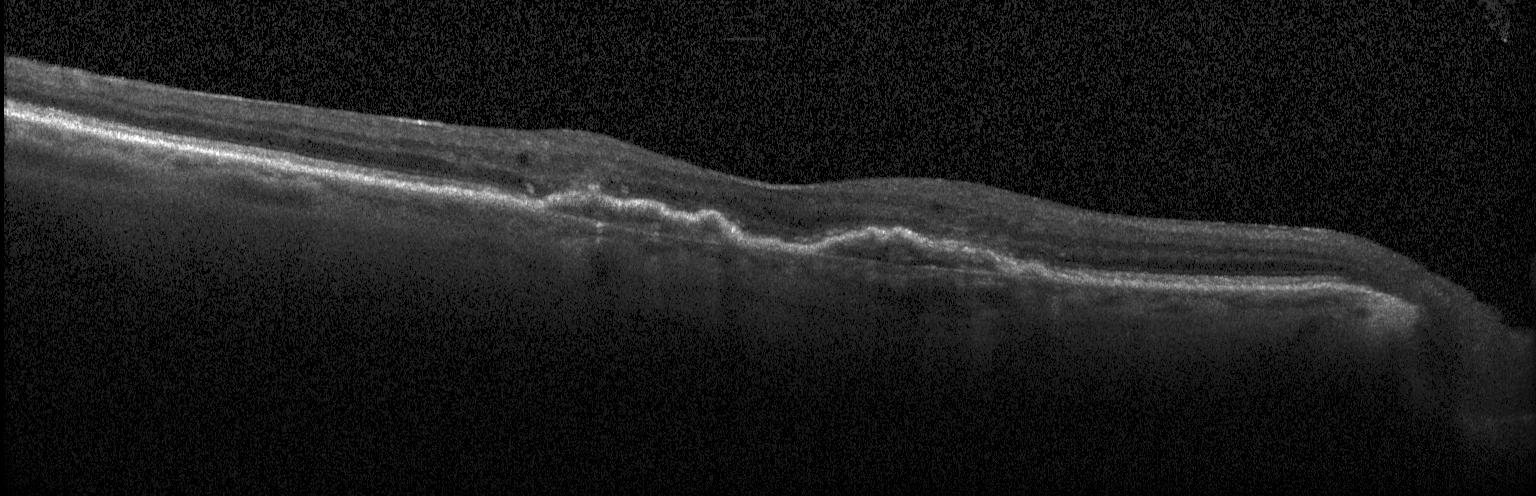
Spectral-domain OCT B-scan: choroidal neovascularization (CNV).